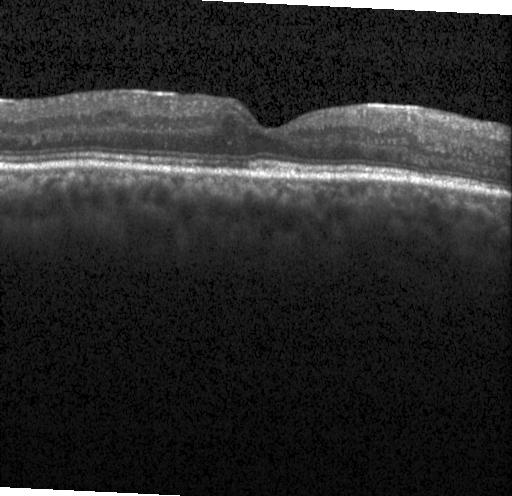
Finding: DME.